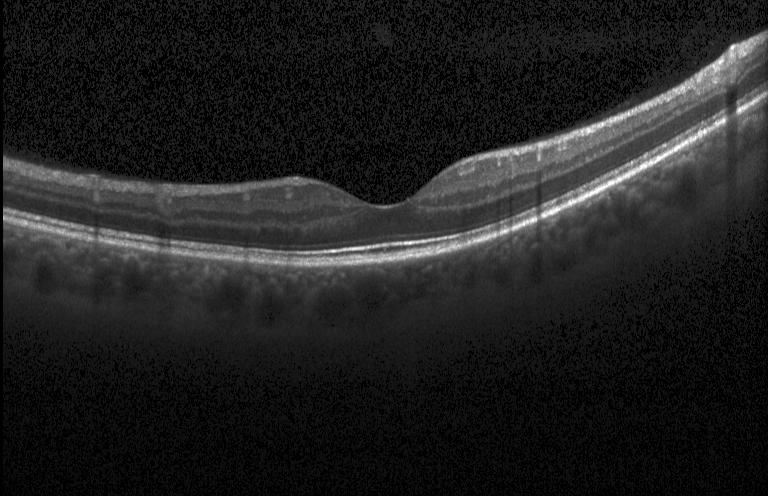 Heidelberg Spectralis OCT system, fovea-centered, optical coherence tomography B-scan, SD-OCT — Diagnosis: no evidence of CNV, DME, or drusen.